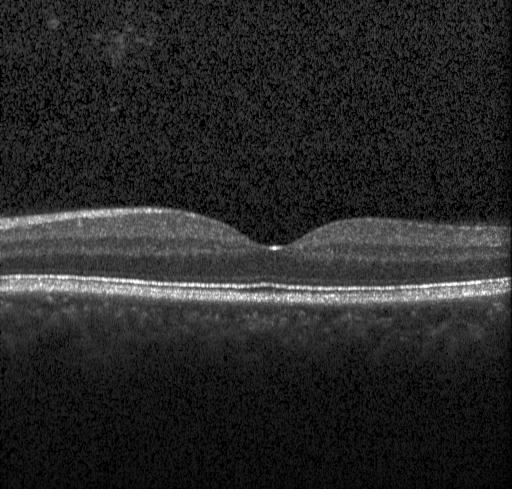 Finding: neither CNV, DME, nor drusen.